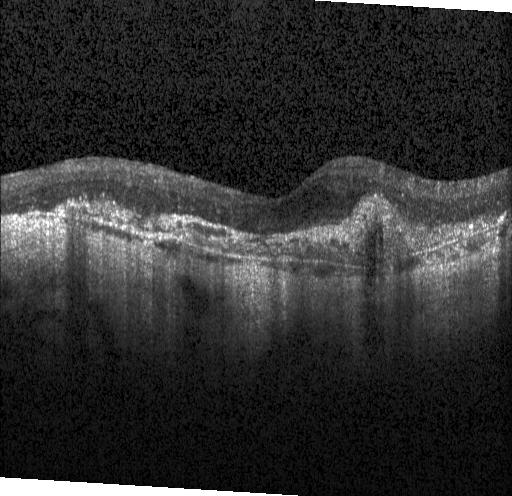
OCT B-scan showing CNV.